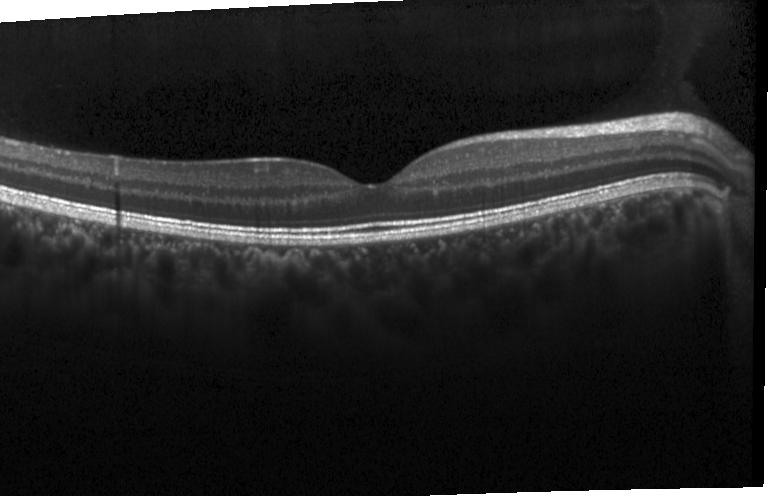 Retinal OCT B-scan.
Impression: no CNV, no DME, and no drusen.